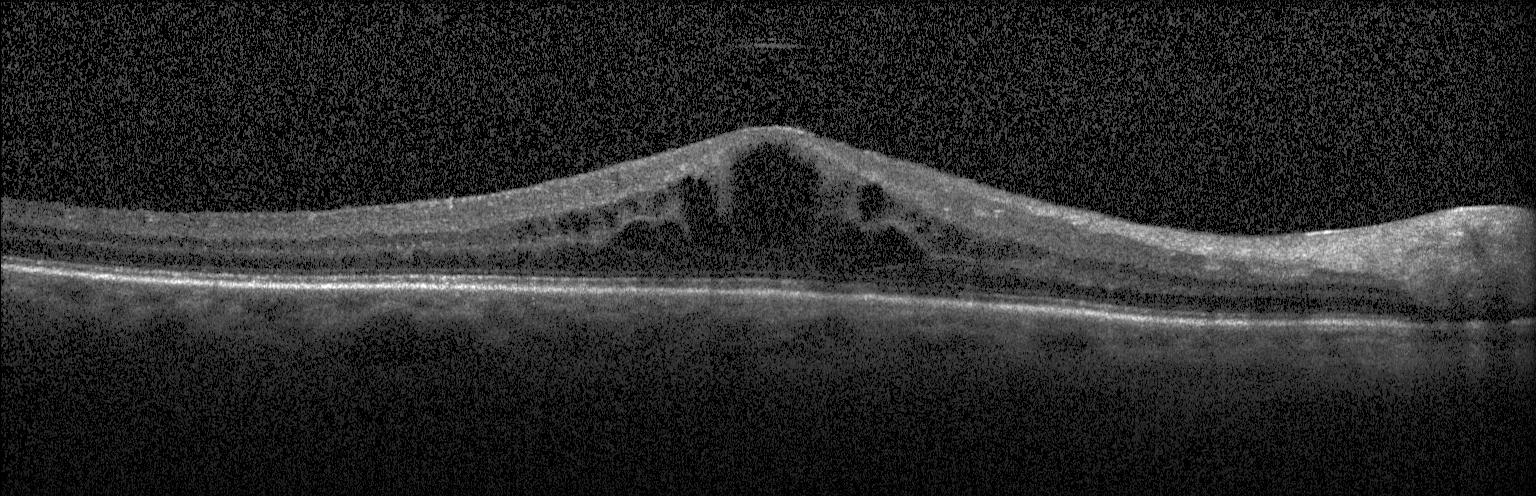 Macular scan. Heidelberg Spectralis. Spectral-domain optical coherence tomography. OCT line scan. Macular OCT: DME.